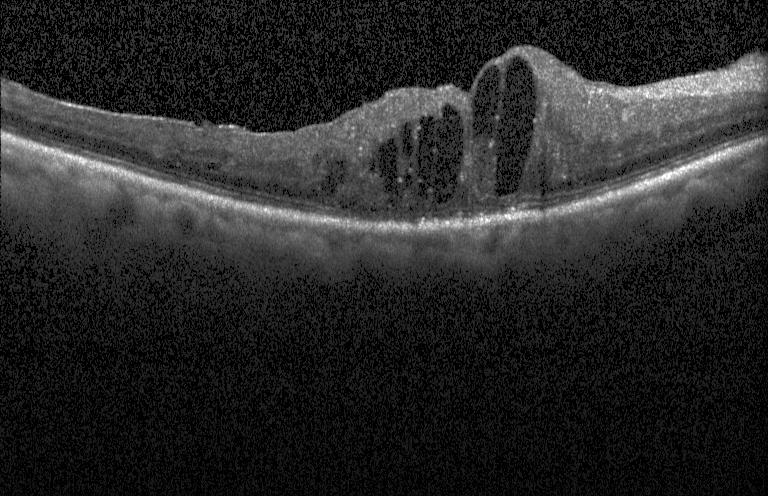 Instrument: Heidelberg Spectralis; optical coherence tomography scan; macular scan; spectral-domain OCT. OCT finding: diabetic macular edema (DME).